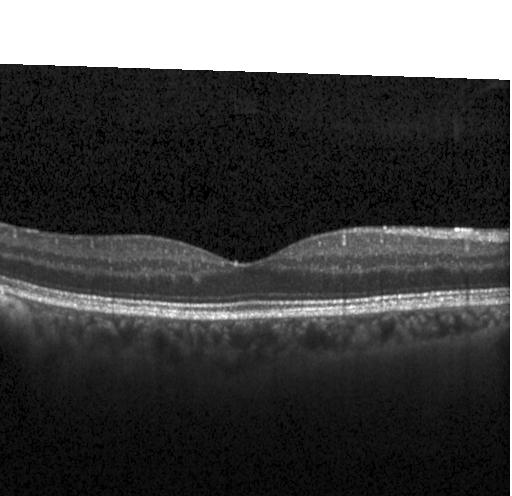 Spectral-domain OCT B-scan: no choroidal neovascularization, no diabetic macular edema, and no drusen.